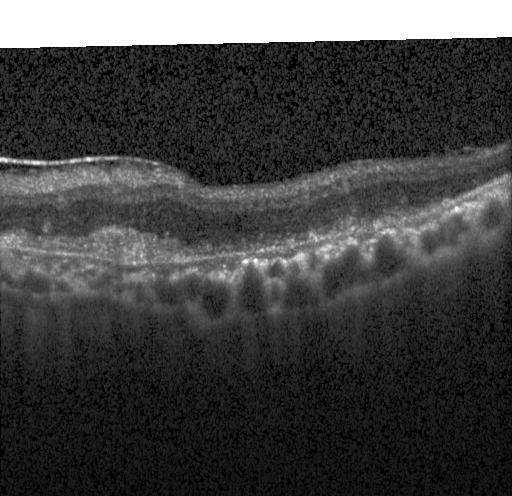

Retinal OCT cross-section showing a choroidal neovascular membrane.